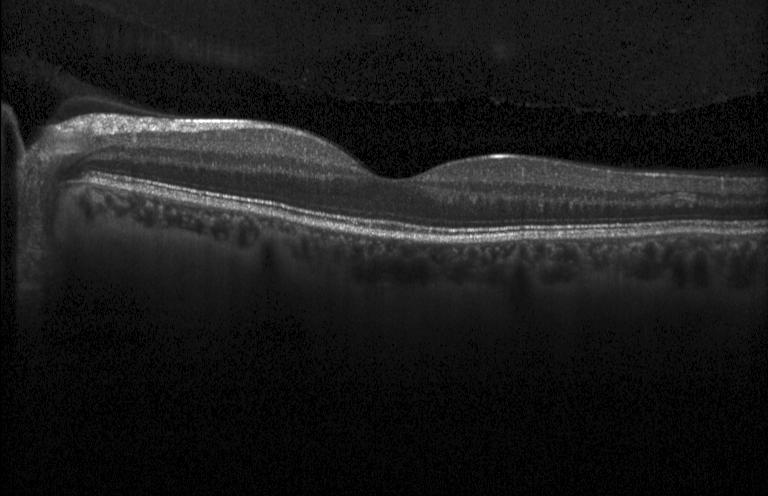
Optical coherence tomography B-scan; Heidelberg Spectralis OCT system; through the macula — This B-scan demonstrates neither choroidal neovascularization, diabetic macular edema, nor drusen.